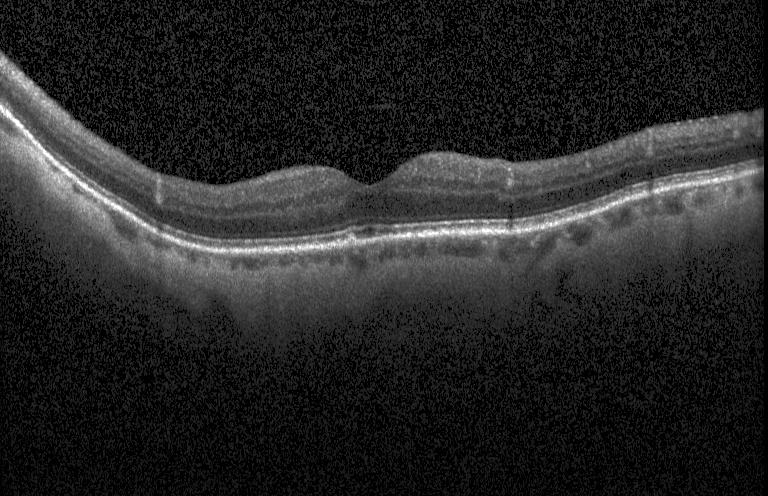 OCT B-scan, instrument: Heidelberg Spectralis. Finding: multiple drusen.